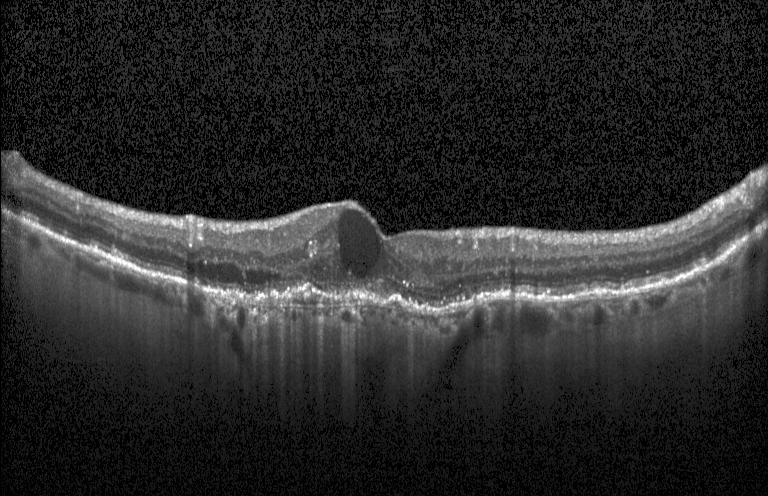
Retinal OCT B-scan. Acquired on a Heidelberg Spectralis — This B-scan demonstrates a choroidal neovascular membrane.